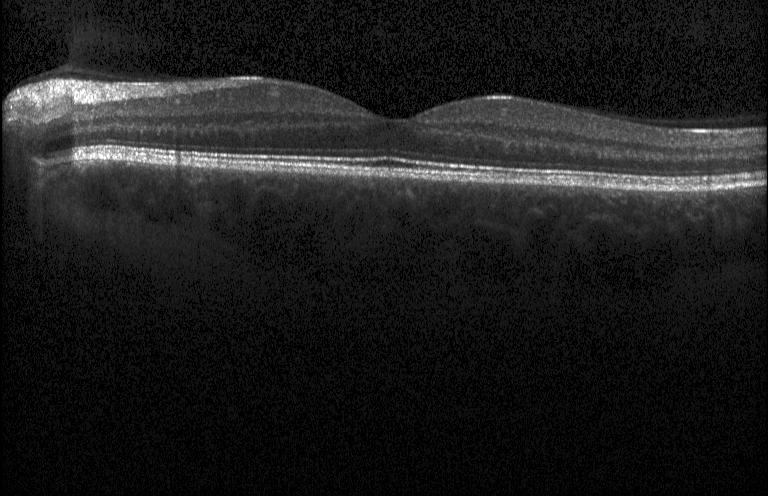
Heidelberg Spectralis; OCT B-scan — This B-scan demonstrates no choroidal neovascularization, diabetic macular edema, or drusen.